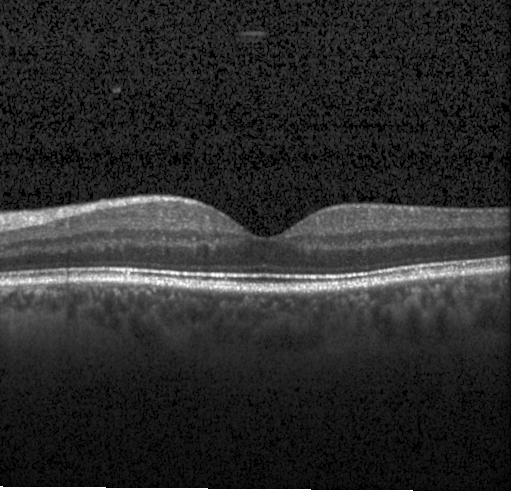

Acquired on a Heidelberg Spectralis, optical coherence tomography B-scan — Macular OCT: no choroidal neovascularization, no diabetic macular edema, and no drusen.